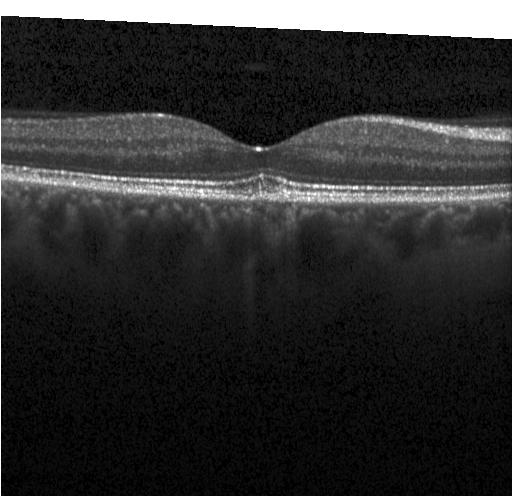

OCT scan showing no evidence of choroidal neovascularization, diabetic macular edema, or drusen.